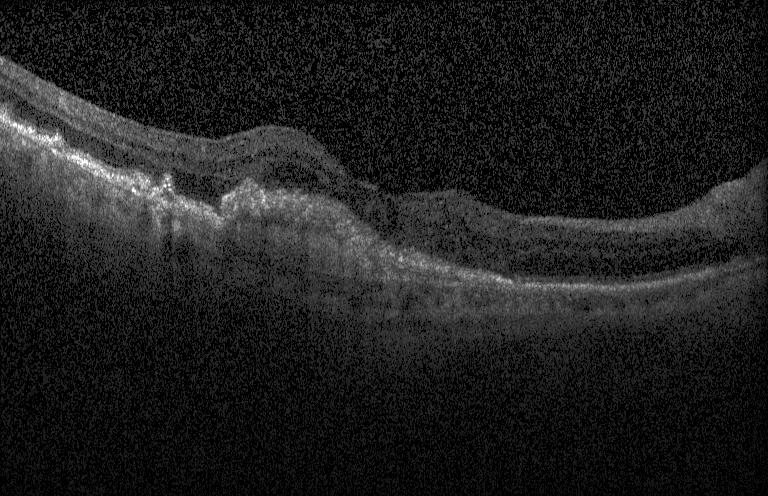 Optical coherence tomography B-scan; spectral-domain OCT. Assessment: CNV.